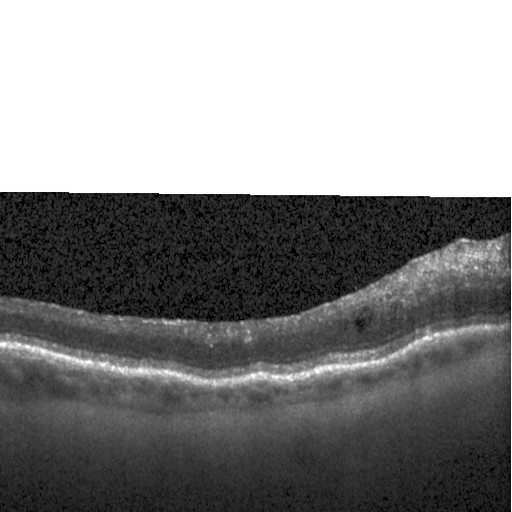 Optical coherence tomography B-scan. The scan shows DME.